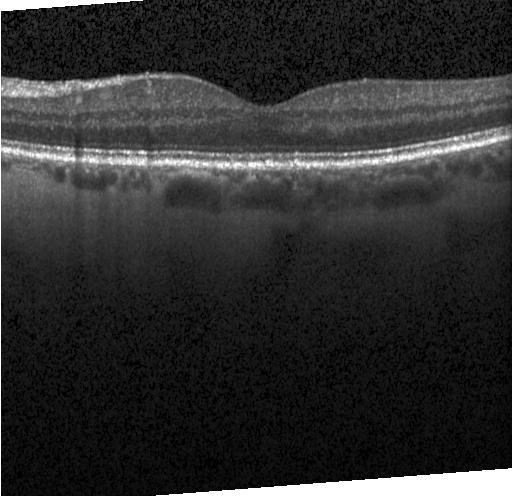 Spectral-domain OCT B-scan: no evidence of CNV, DME, or drusen.